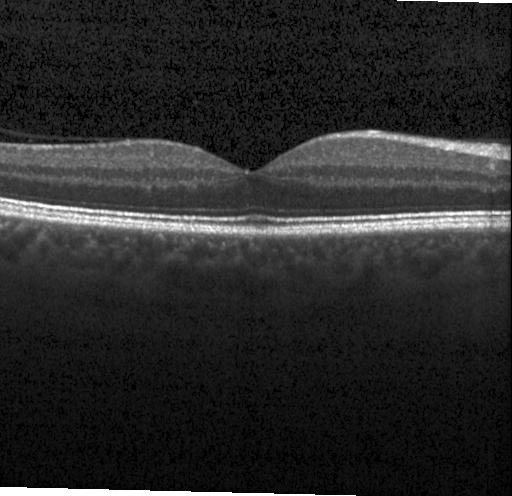
OCT line scan.
Diagnosis: no evidence of CNV, DME, or drusen.